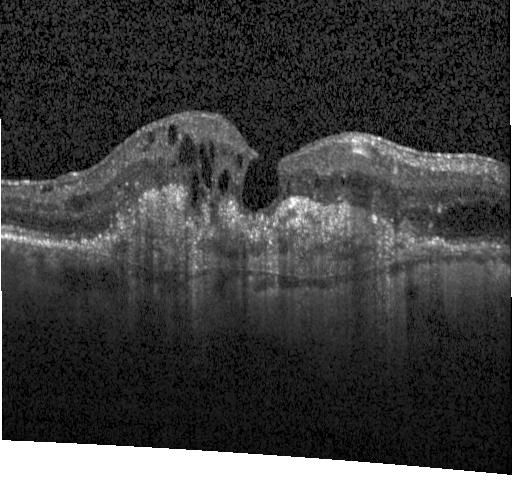
This B-scan demonstrates choroidal neovascularization.